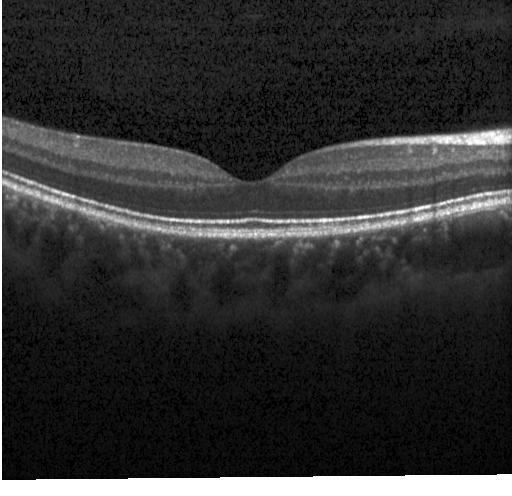

Retinal OCT cross-section. Finding: no evidence of CNV, DME, or drusen.